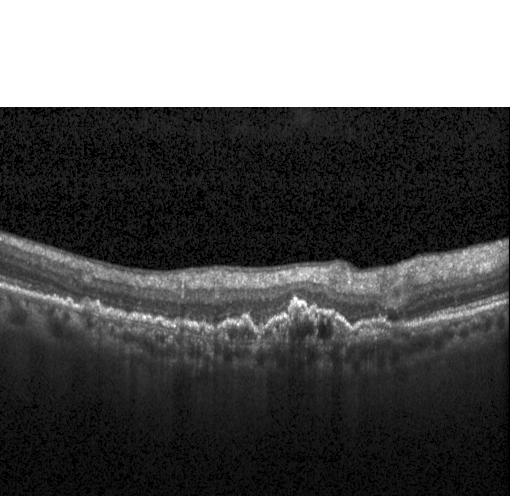
Finding: CNV.